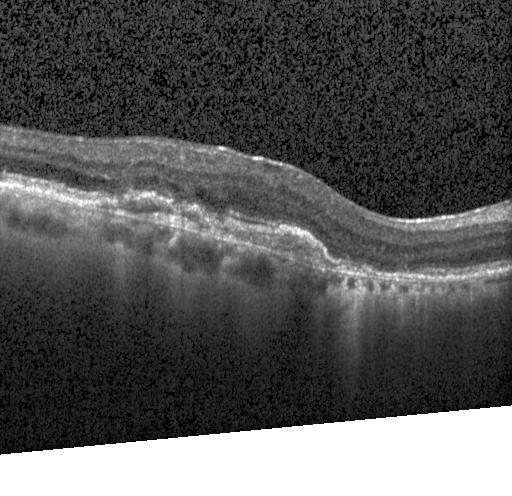
Optical coherence tomography scan — The scan shows a choroidal neovascular membrane.